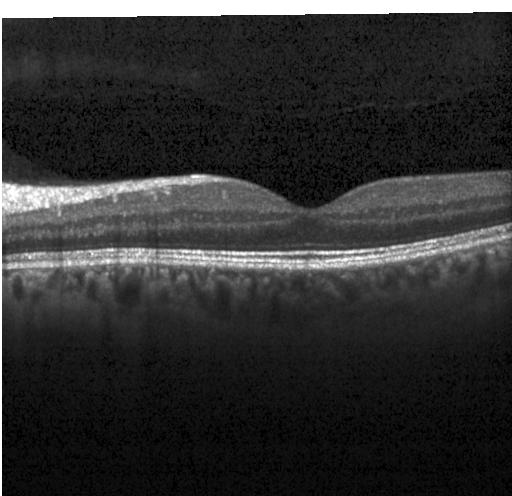
Optical coherence tomography scan · horizontal scan through the fovea · instrument: Heidelberg Spectralis — Dx: no evidence of CNV, DME, or drusen.